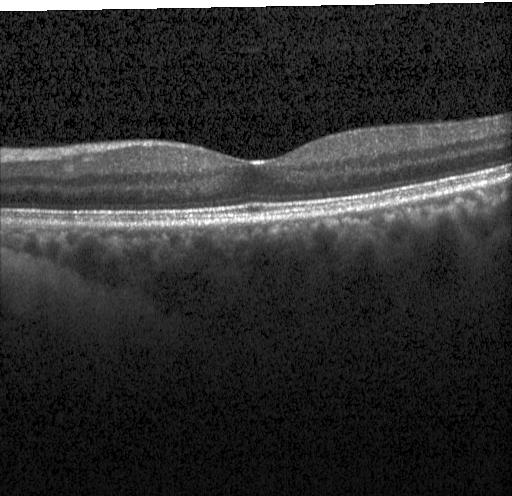
Heidelberg Spectralis OCT system · optical coherence tomography B-scan · through the macula
This B-scan demonstrates no CNV, DME, or drusen.